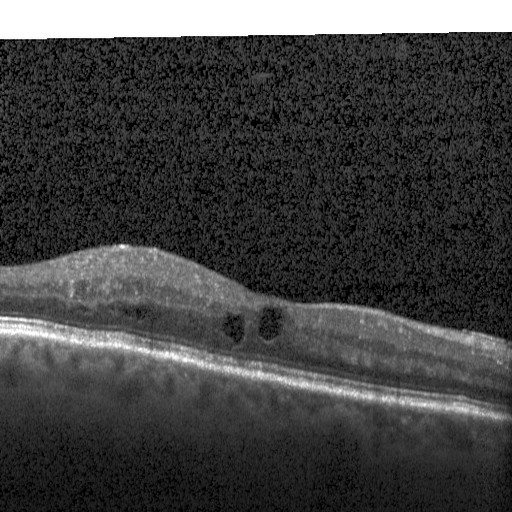

The scan shows diabetic macular edema.